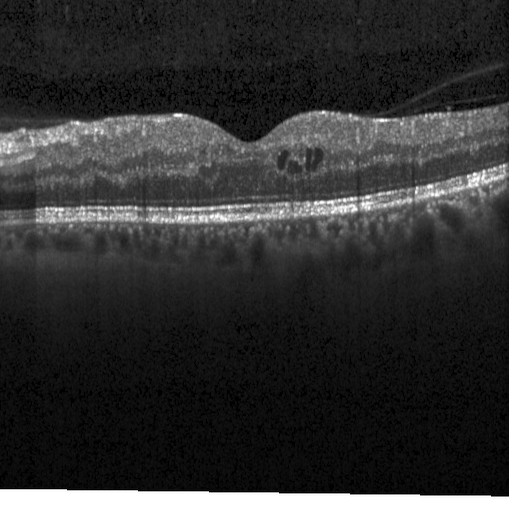 Macular OCT demonstrating diabetic macular edema.